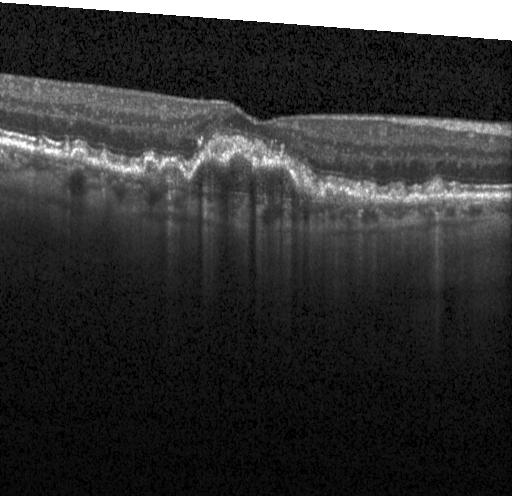 Assessment: CNV.